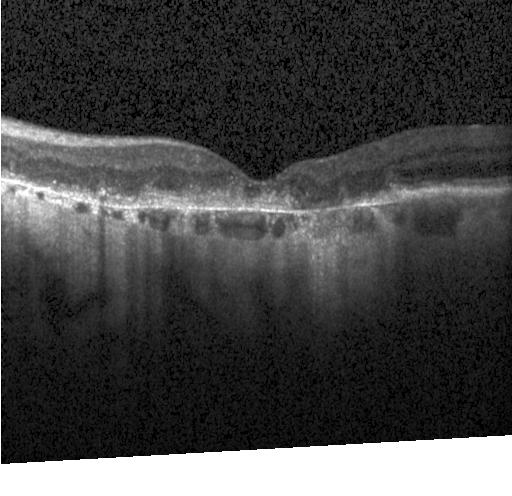 Optical coherence tomography scan.
Macular OCT: a choroidal neovascular membrane.